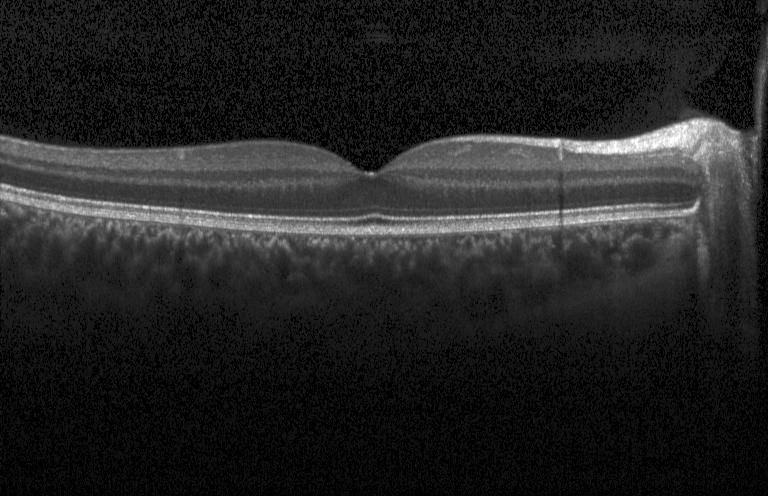 Retinal OCT cross-section — Macular OCT: no evidence of choroidal neovascularization, diabetic macular edema, or drusen.